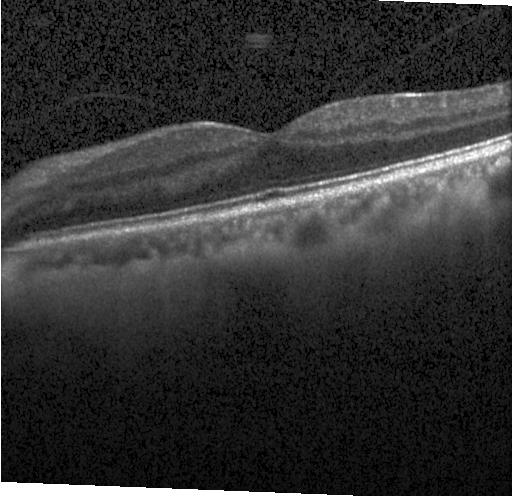
OCT line scan
Finding: neither choroidal neovascularization, diabetic macular edema, nor drusen.